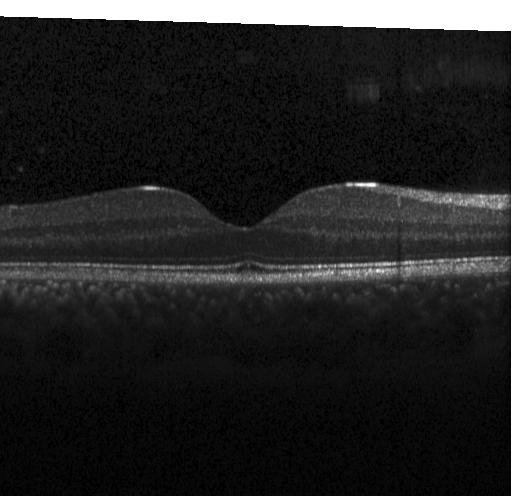
Retinal OCT B-scan.
This B-scan demonstrates neither choroidal neovascularization, diabetic macular edema, nor drusen.